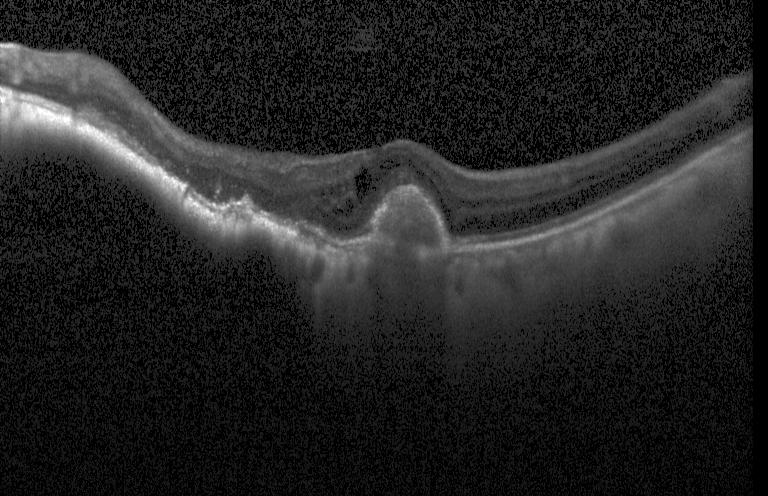

Optical coherence tomography scan · Heidelberg Spectralis OCT system
Impression: a choroidal neovascular membrane.